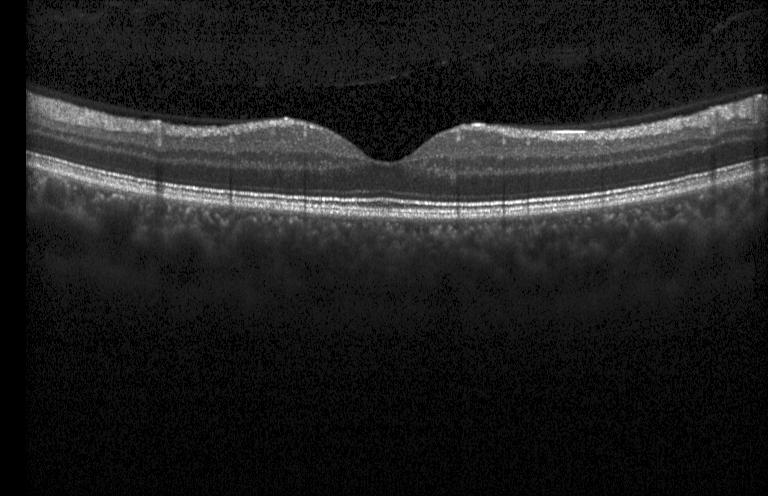

No CNV, no DME, and no drusen.